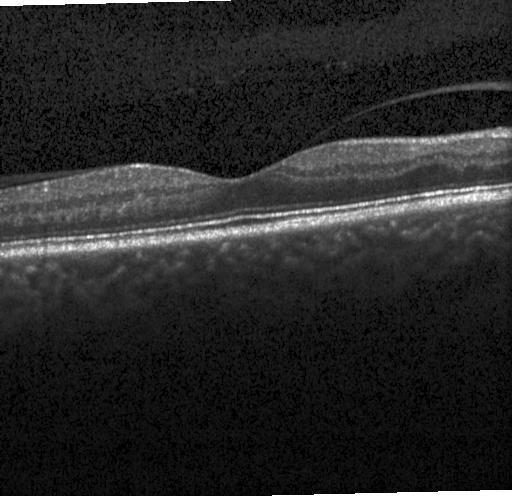

SD-OCT. OCT B-scan — This B-scan demonstrates no choroidal neovascularization, diabetic macular edema, or drusen.